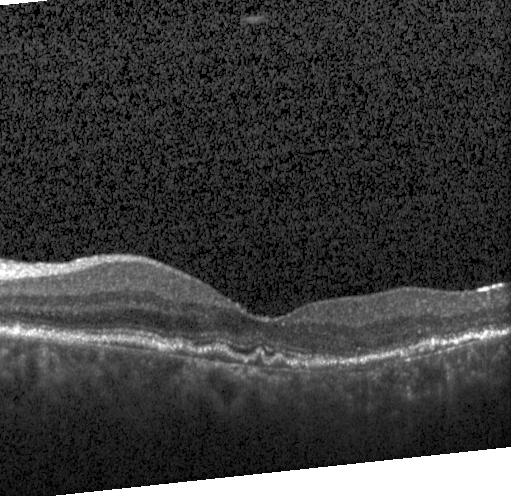
Centered on the fovea, OCT B-scan, instrument: Heidelberg Spectralis — Diagnosis: choroidal neovascularization (CNV).